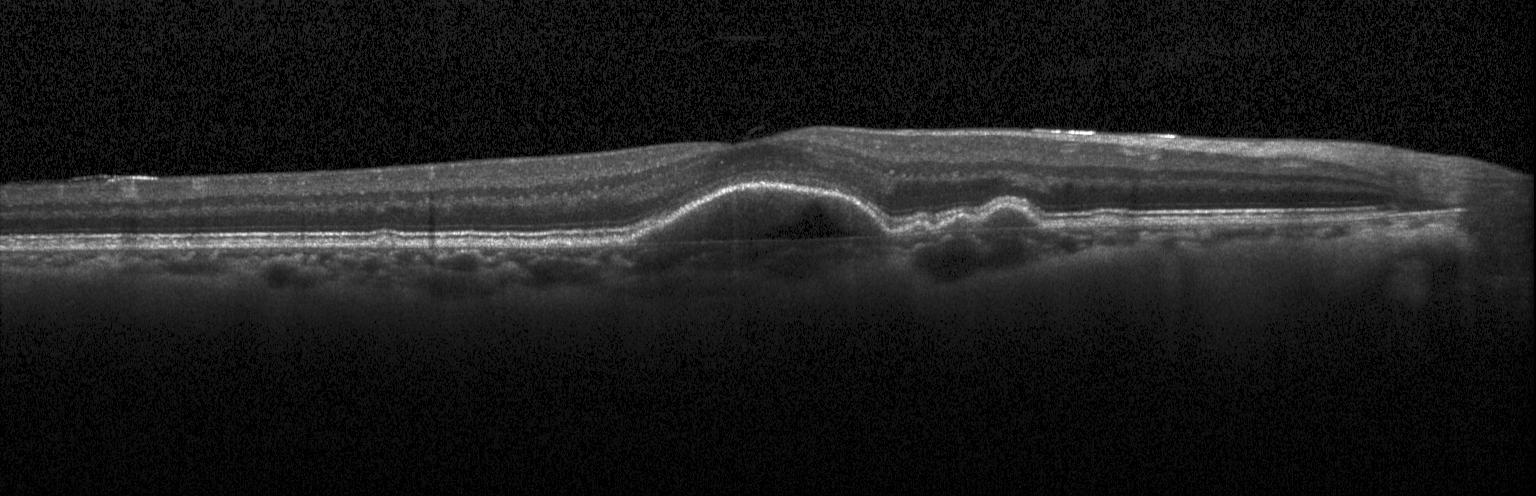
OCT B-scan showing choroidal neovascularization (CNV).